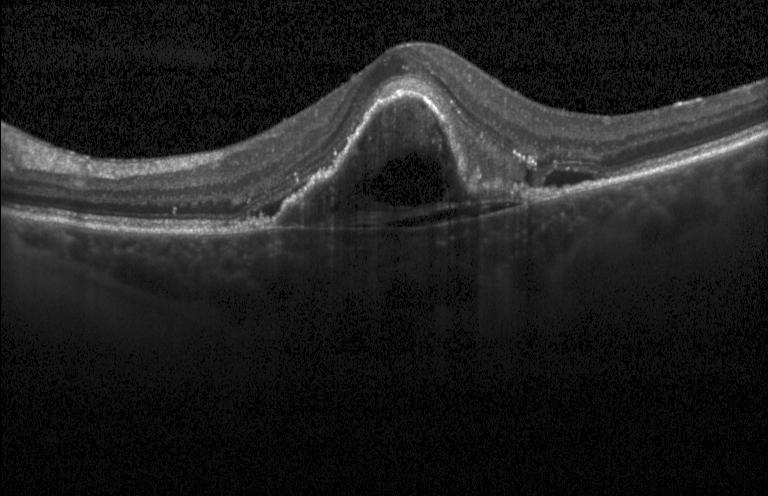 Impression: a choroidal neovascular membrane.